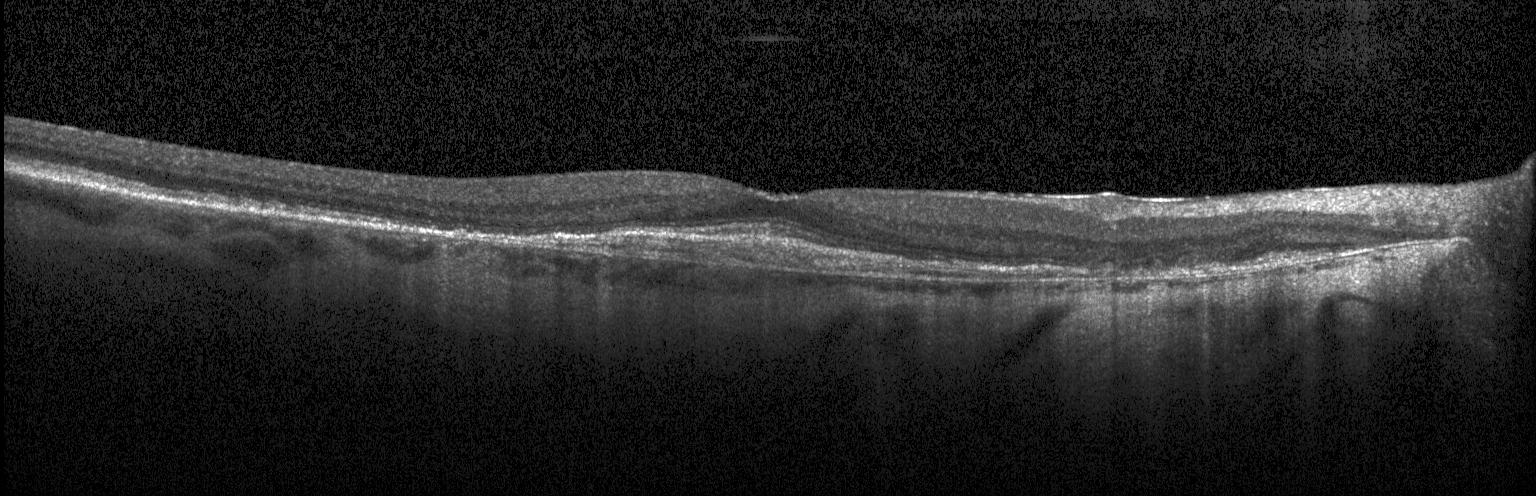

OCT finding: a choroidal neovascular membrane.